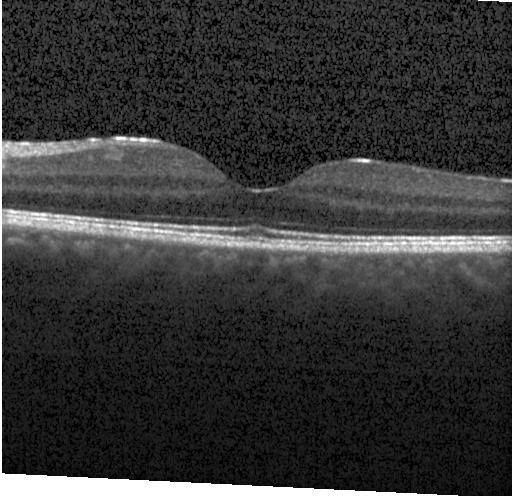 Macular scan · retinal OCT B-scan · spectral-domain OCT. The scan shows no CNV, no DME, and no drusen.